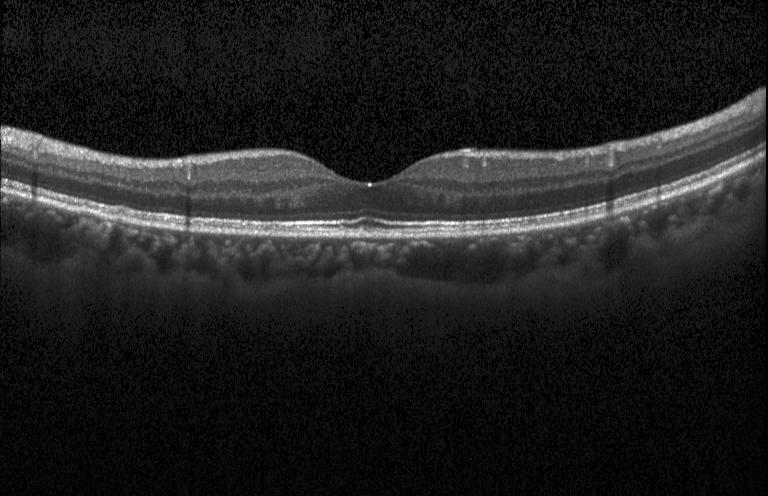 OCT B-scan. Heidelberg Spectralis — This B-scan demonstrates no evidence of CNV, DME, or drusen.